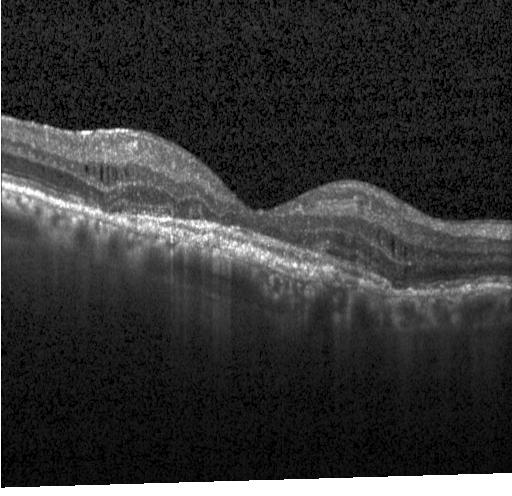

Finding: a choroidal neovascular membrane.